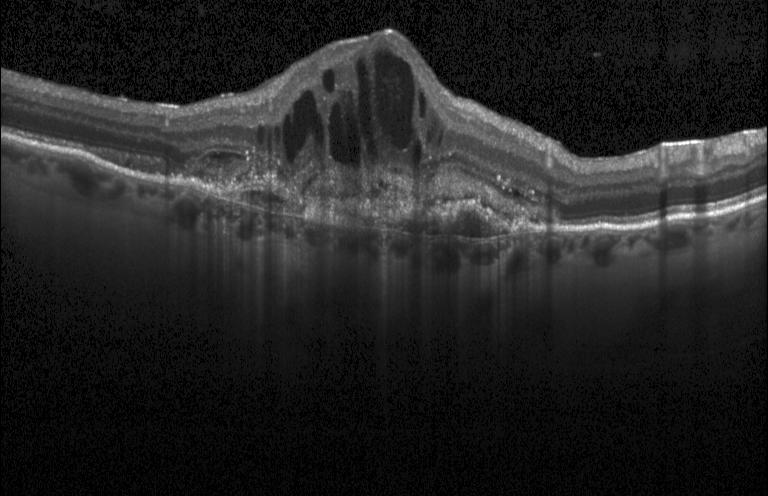 OCT scan showing a choroidal neovascular membrane.